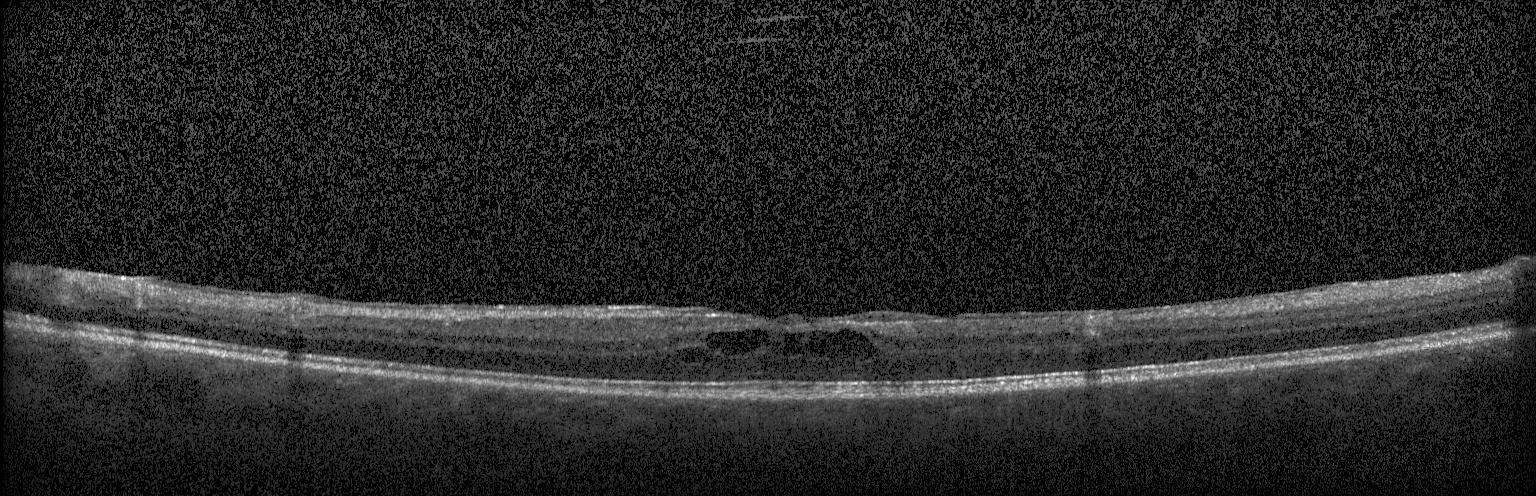 OCT B-scan. SD-OCT. Centered on the fovea. Instrument: Heidelberg Spectralis.
Impression: DME.